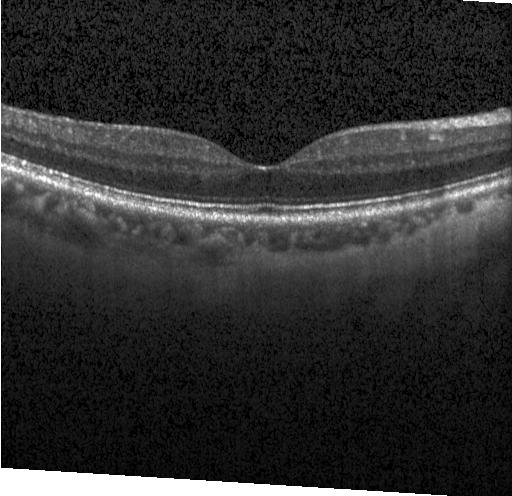
Spectral-domain optical coherence tomography. Retinal OCT cross-section. Acquired on a Heidelberg Spectralis
OCT finding: no evidence of CNV, DME, or drusen.